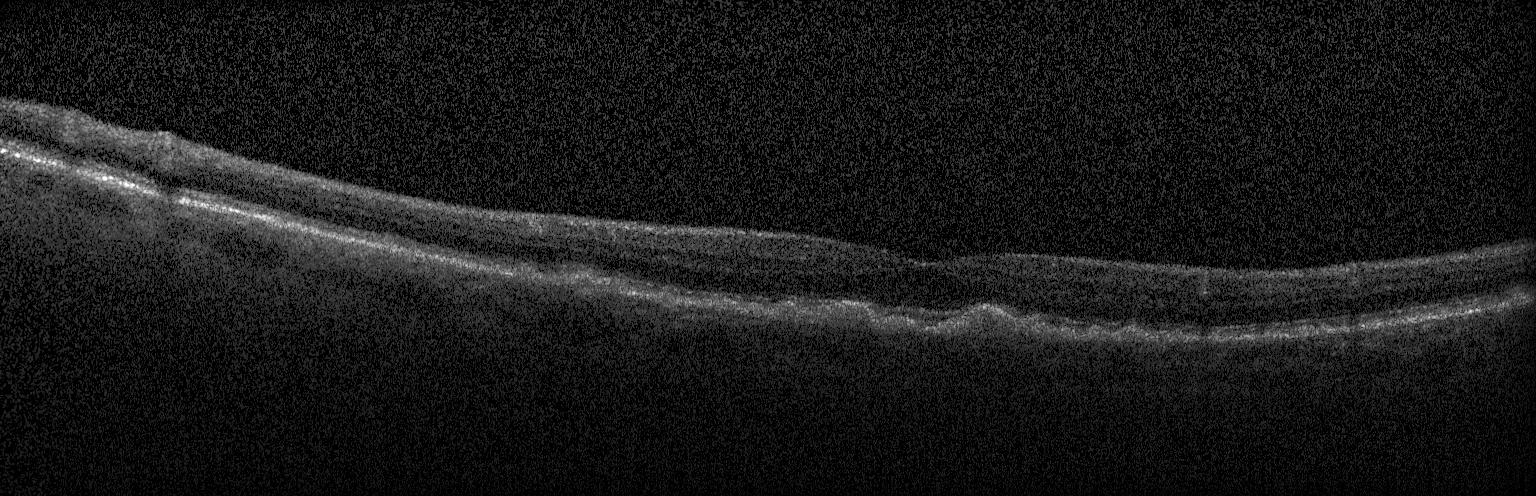
Horizontal scan through the fovea · SD-OCT · retinal OCT cross-section · Heidelberg Spectralis — Finding: drusen.